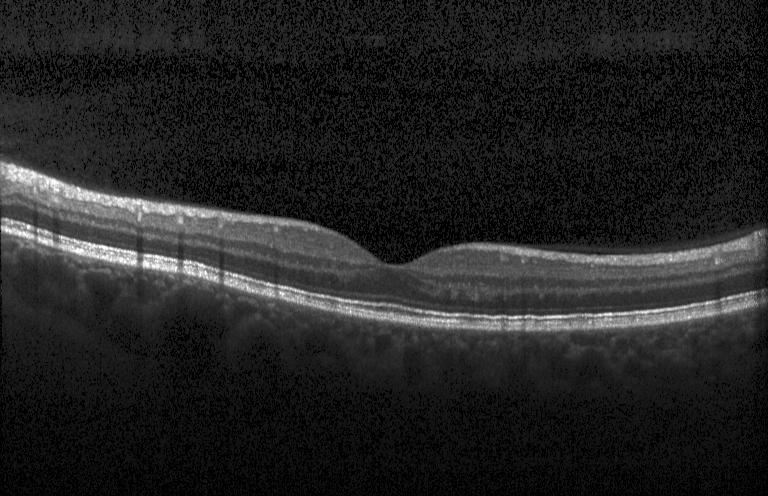
Spectral-domain OCT B-scan: no choroidal neovascularization, no diabetic macular edema, and no drusen.